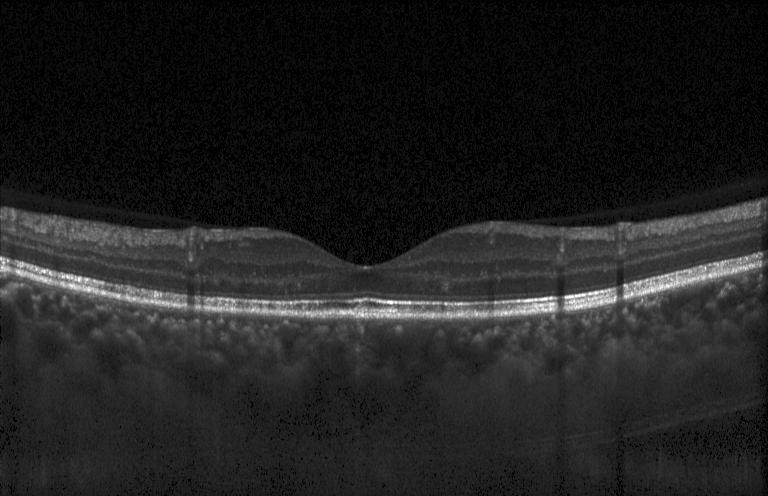
Centered on the fovea, acquired on a Heidelberg Spectralis, SD-OCT, optical coherence tomography scan.
This B-scan demonstrates no CNV, DME, or drusen.